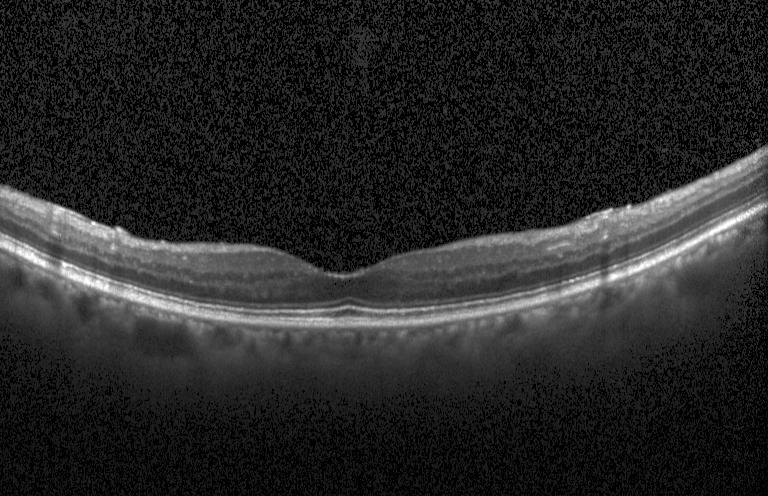
Finding: no choroidal neovascularization, diabetic macular edema, or drusen.